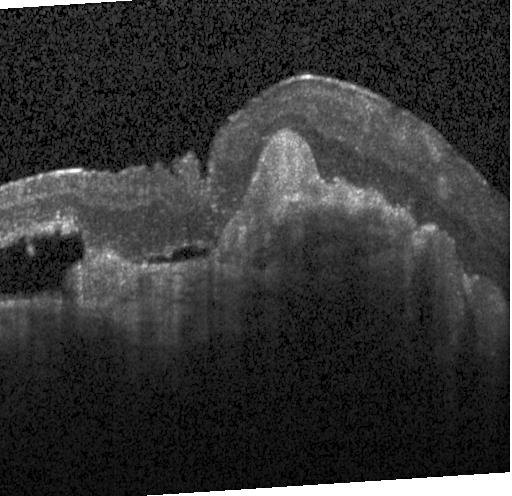 Retinal OCT cross-section showing choroidal neovascularization.